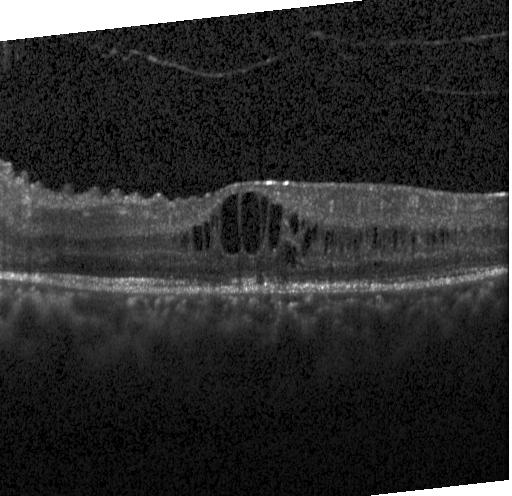

OCT B-scan showing diabetic macular edema (DME).